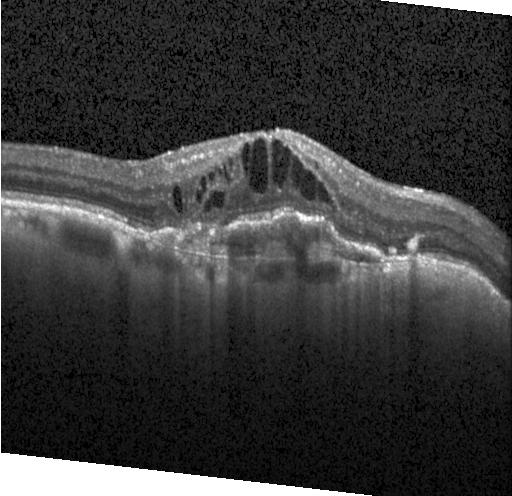 Assessment: choroidal neovascularization.